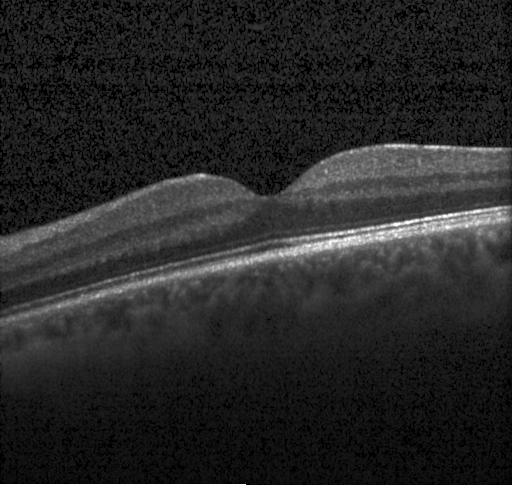 No choroidal neovascularization, no diabetic macular edema, and no drusen.